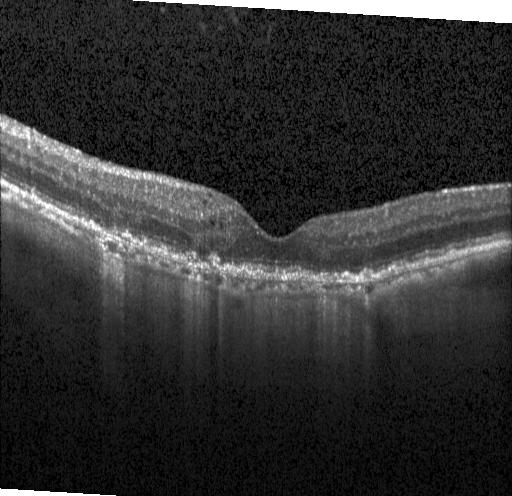
Acquired on a Heidelberg Spectralis. SD-OCT. Optical coherence tomography scan. Dx: a choroidal neovascular membrane.